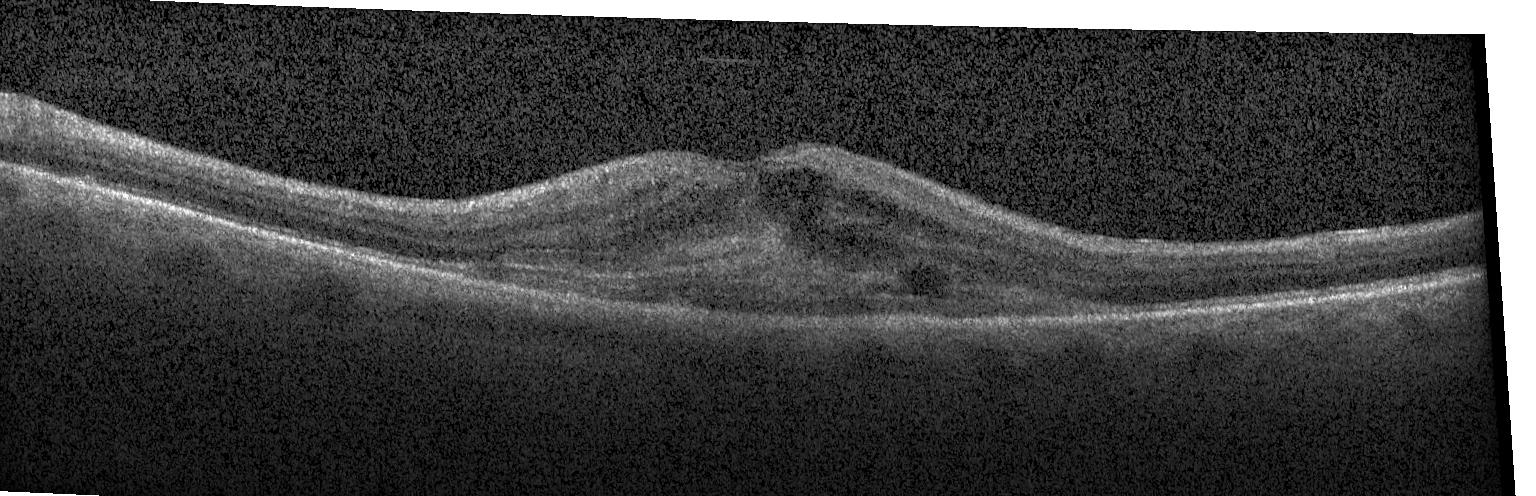
Retinal OCT cross-section; SD-OCT; Heidelberg Spectralis OCT system; macular scan. Diagnosis: choroidal neovascularization (CNV).